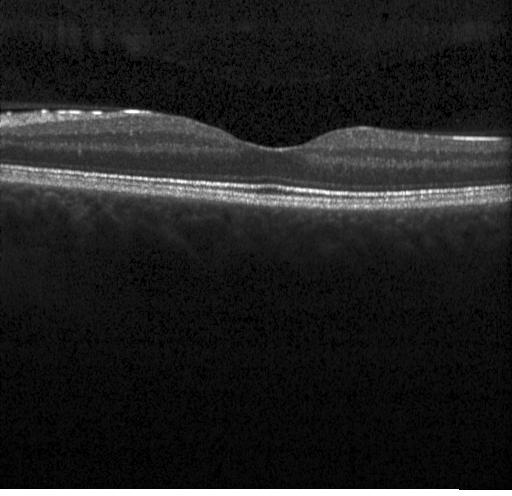
Centered on the fovea; Heidelberg Spectralis; spectral-domain OCT; OCT B-scan.
Assessment: no evidence of choroidal neovascularization, diabetic macular edema, or drusen.